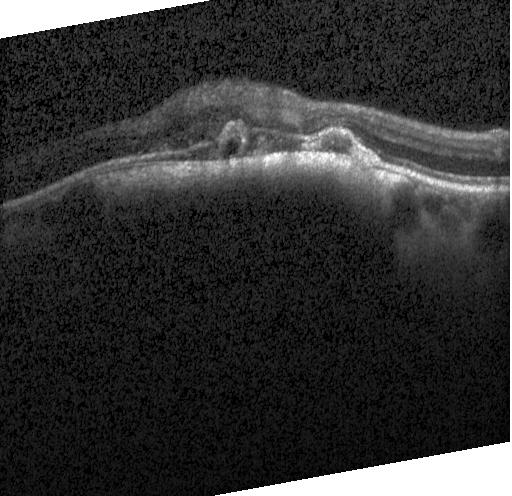

OCT B-scan.
Assessment: choroidal neovascularization (CNV).